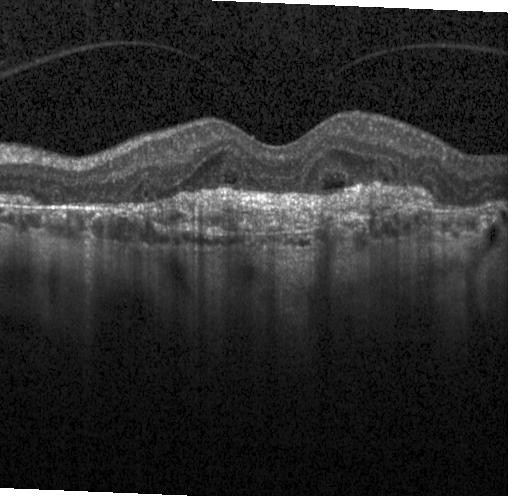
Retinal OCT cross-section
Impression: choroidal neovascularization (CNV).